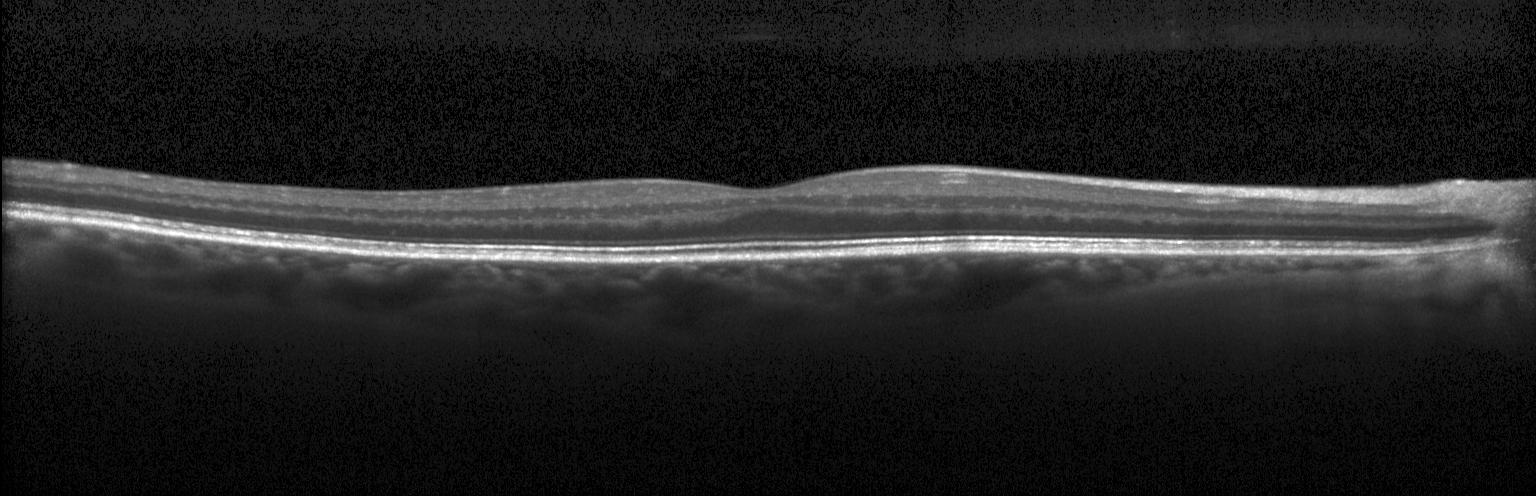

Macular OCT: neither choroidal neovascularization, diabetic macular edema, nor drusen.